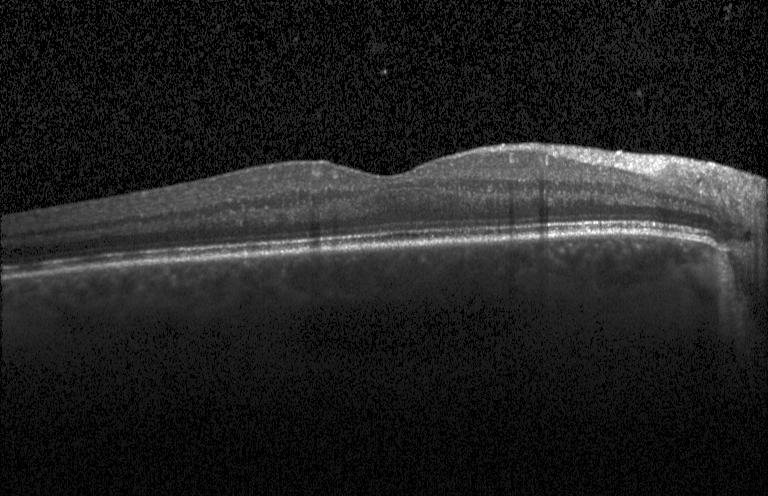
Spectral-domain OCT, Heidelberg Spectralis OCT system, optical coherence tomography scan, fovea-centered. Assessment: no evidence of choroidal neovascularization, diabetic macular edema, or drusen.